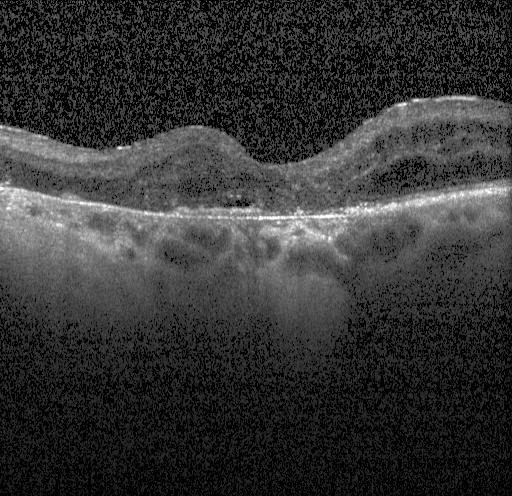

Spectral-domain OCT. Optical coherence tomography scan. Assessment: a choroidal neovascular membrane.